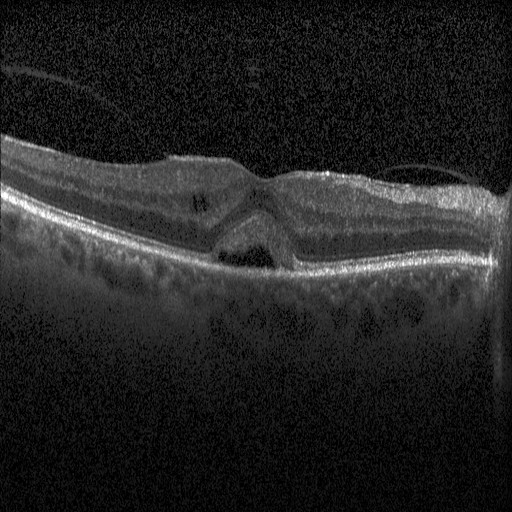
Impression: diabetic macular edema (DME).